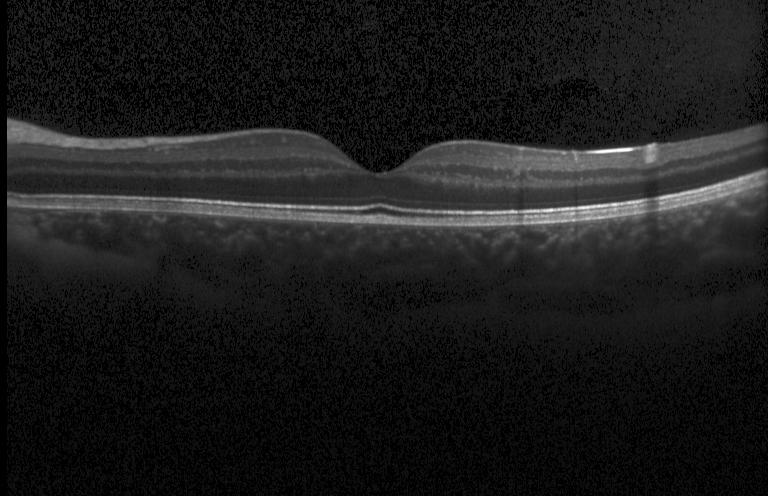 Centered on the fovea, retinal OCT B-scan
Finding: no evidence of choroidal neovascularization, diabetic macular edema, or drusen.